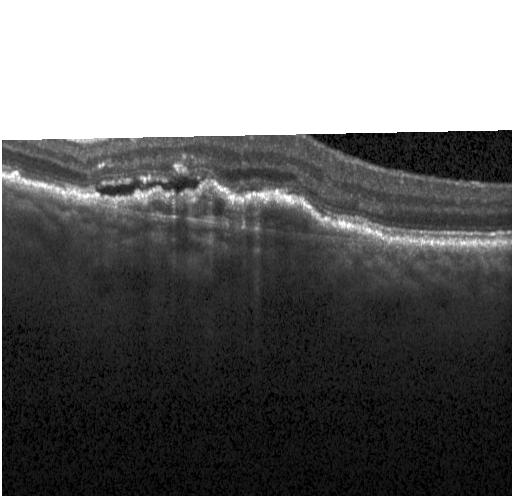

Optical coherence tomography scan, SD-OCT, macular scan. OCT finding: a choroidal neovascular membrane.